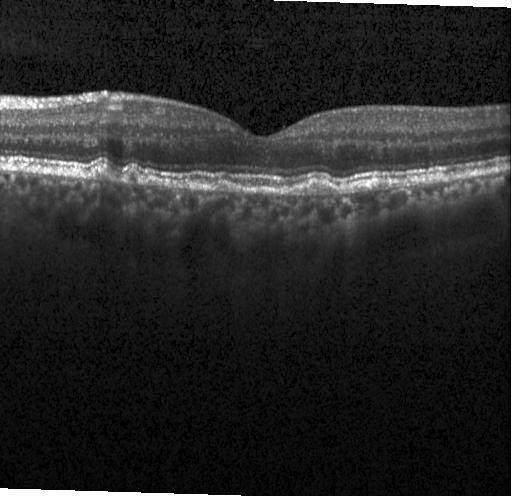

OCT finding: drusen.